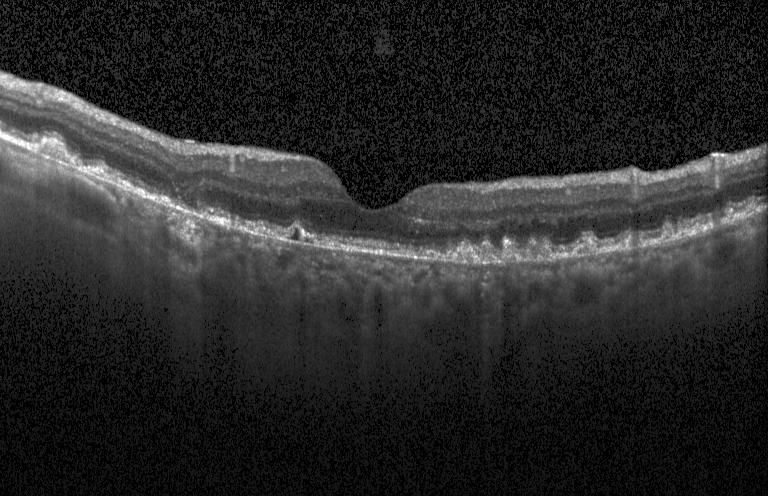

Impression: a choroidal neovascular membrane.